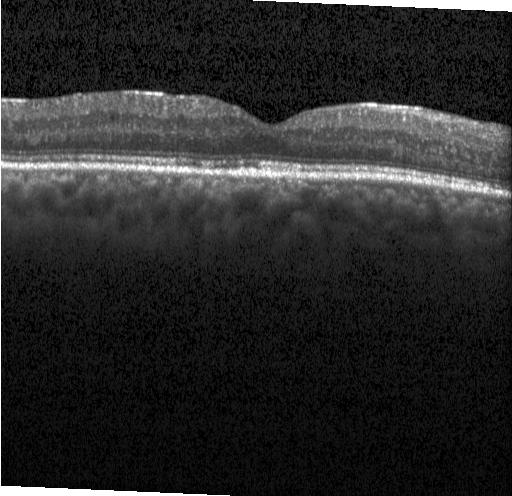
OCT B-scan · Heidelberg Spectralis · fovea-centered — The scan shows no evidence of choroidal neovascularization, diabetic macular edema, or drusen.